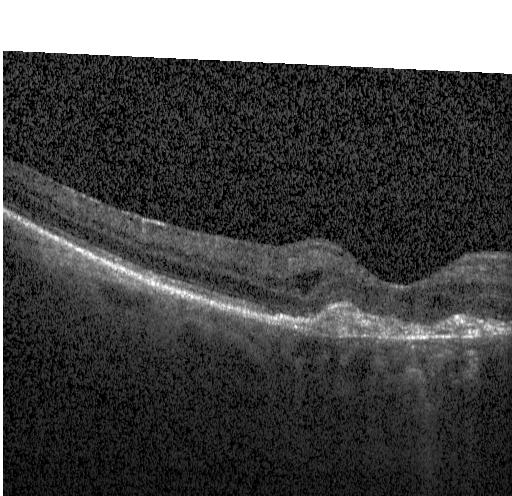
Finding: choroidal neovascularization.